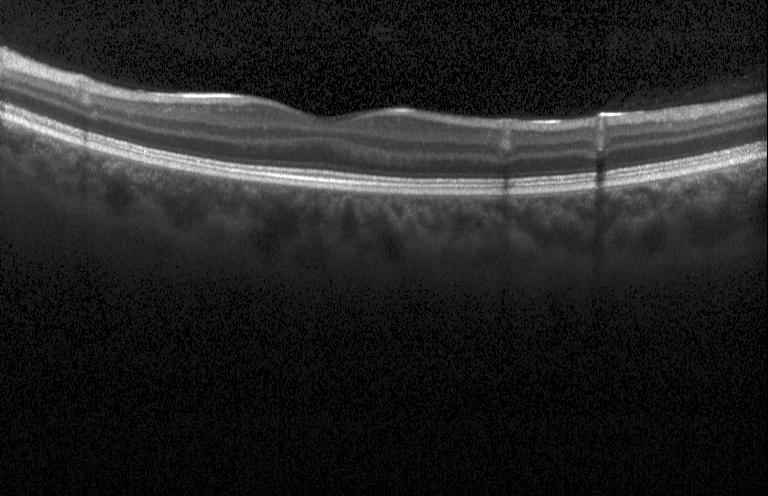

Finding: no choroidal neovascularization, diabetic macular edema, or drusen.